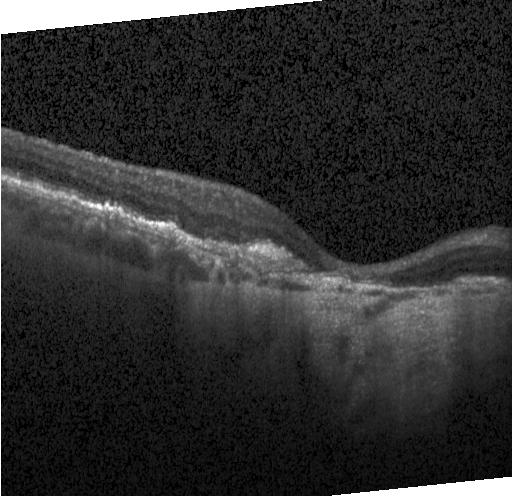

Assessment: a choroidal neovascular membrane.